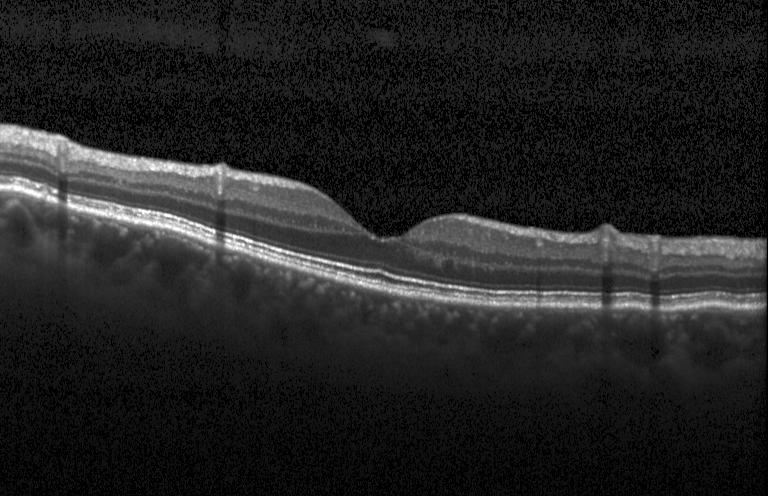
Finding: no evidence of choroidal neovascularization, diabetic macular edema, or drusen.